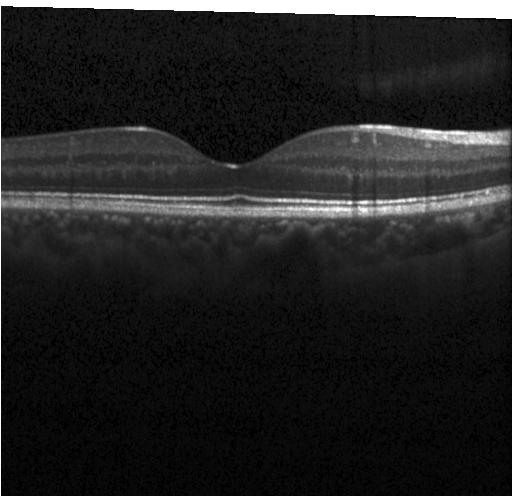
This B-scan demonstrates no CNV, DME, or drusen.